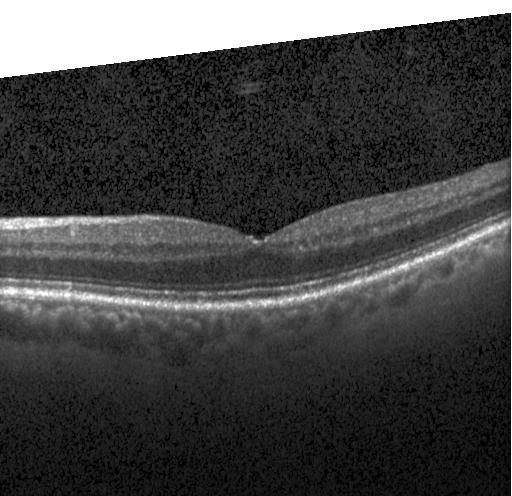
SD-OCT. Retinal OCT cross-section. Acquired on a Heidelberg Spectralis. Macular scan — Impression: no choroidal neovascularization, diabetic macular edema, or drusen.